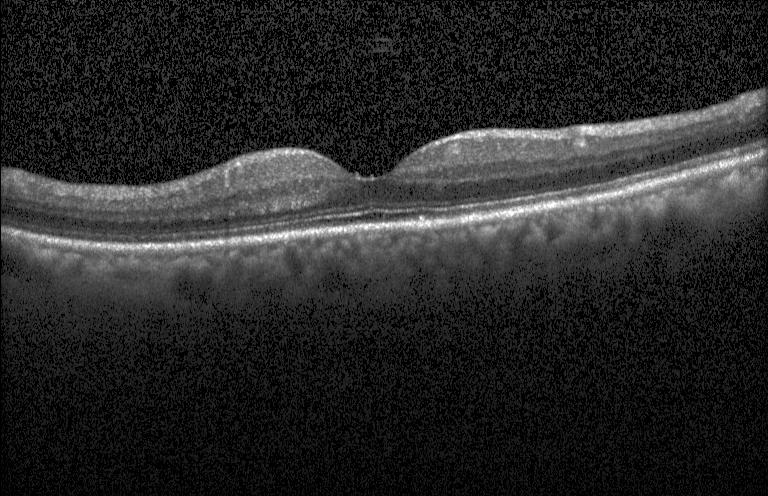
Heidelberg Spectralis OCT system · OCT B-scan · centered on the fovea · SD-OCT. Finding: no evidence of choroidal neovascularization, diabetic macular edema, or drusen.